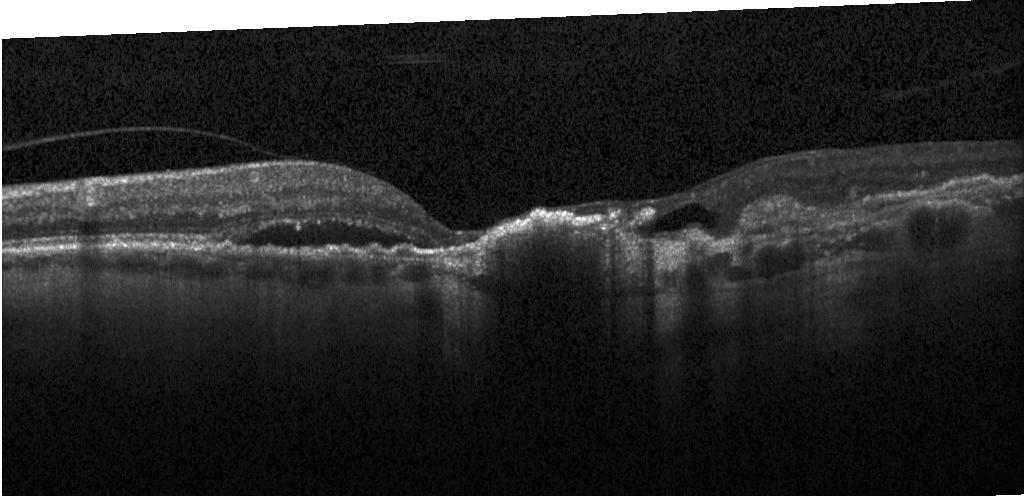

Retinal OCT cross-section; acquired on a Heidelberg Spectralis — Impression: a choroidal neovascular membrane.